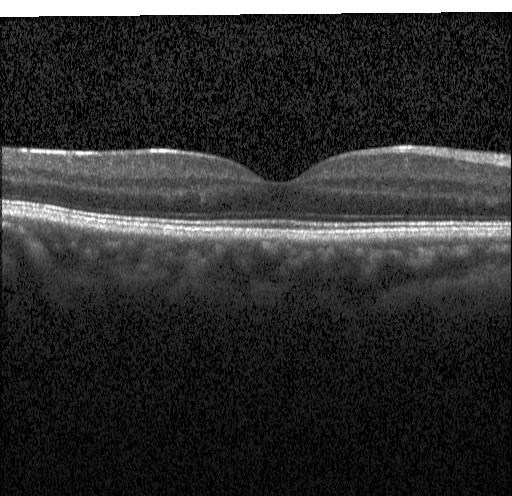 Impression: no CNV, no DME, and no drusen.